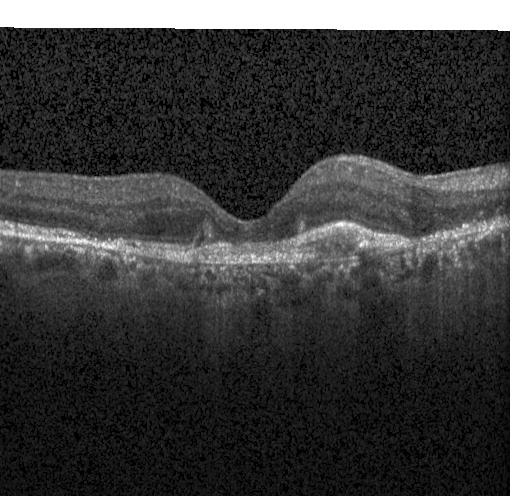 OCT B-scan showing choroidal neovascularization (CNV).